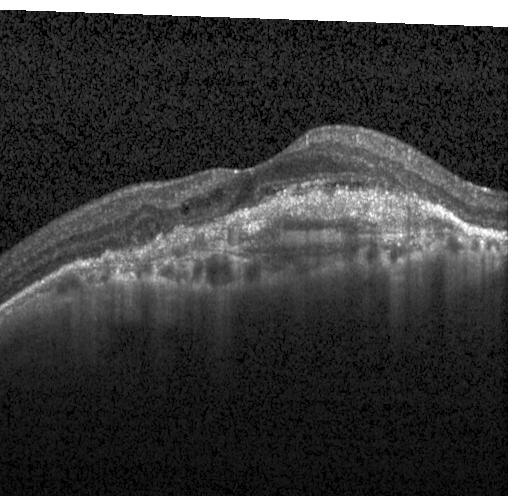
Retinal OCT cross-section showing a choroidal neovascular membrane.